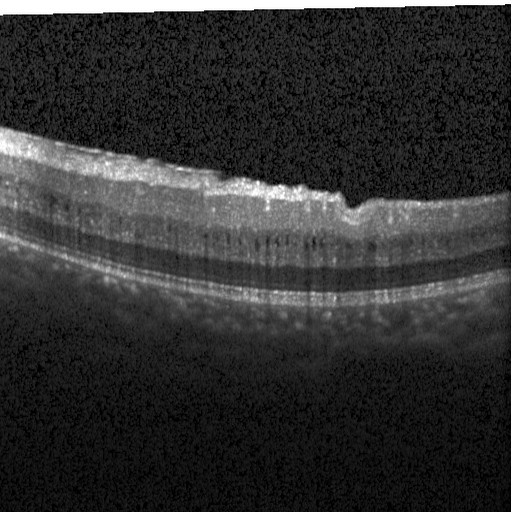
OCT finding: diabetic macular edema.